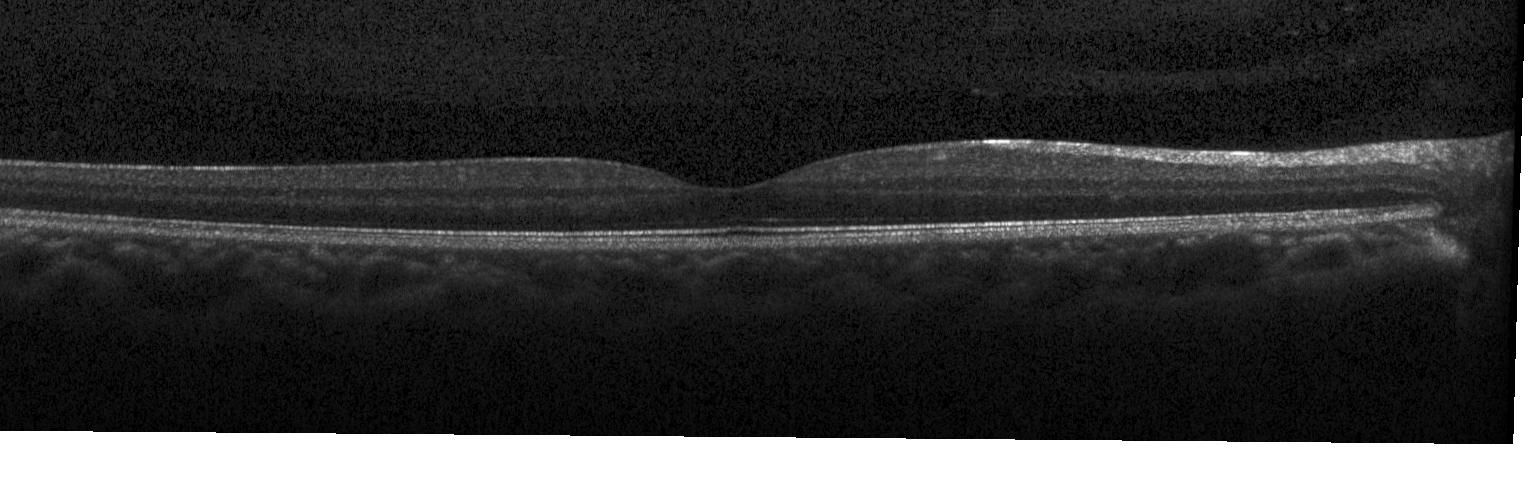 Instrument: Heidelberg Spectralis · retinal OCT cross-section
No evidence of choroidal neovascularization, diabetic macular edema, or drusen.